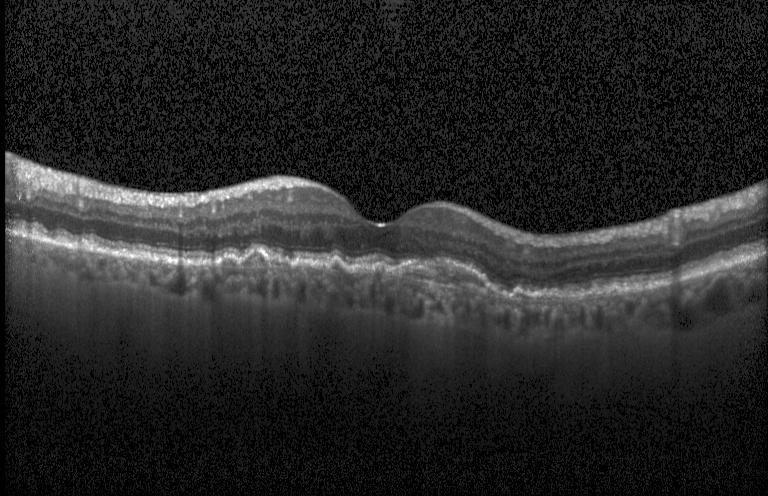 Spectral-domain OCT B-scan: a choroidal neovascular membrane.